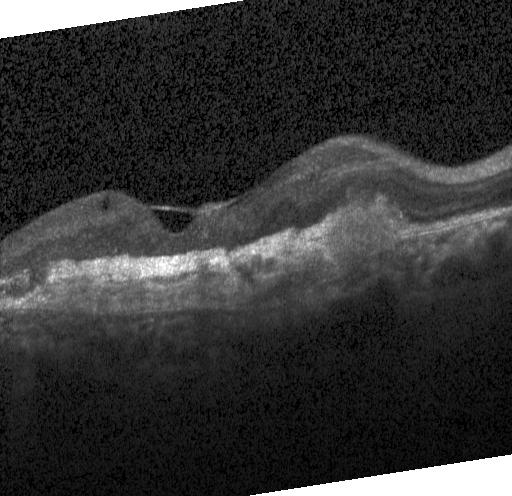

The scan shows a choroidal neovascular membrane.